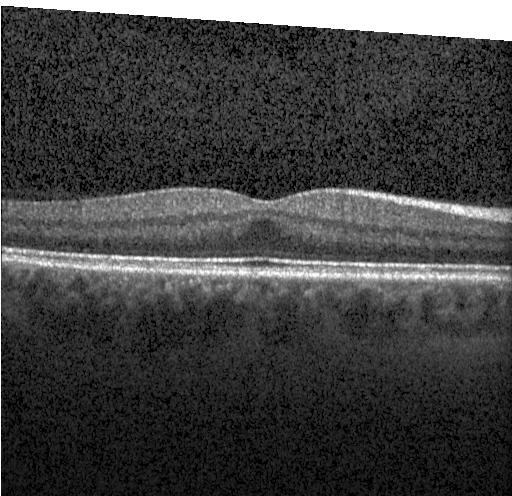 Impression: no evidence of CNV, DME, or drusen.